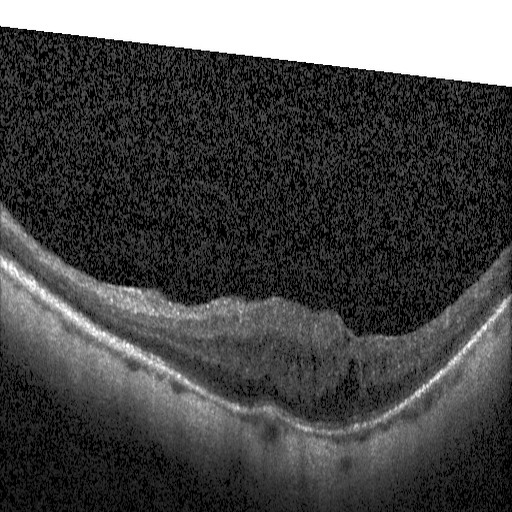 Retinal OCT cross-section · fovea-centered. DME.